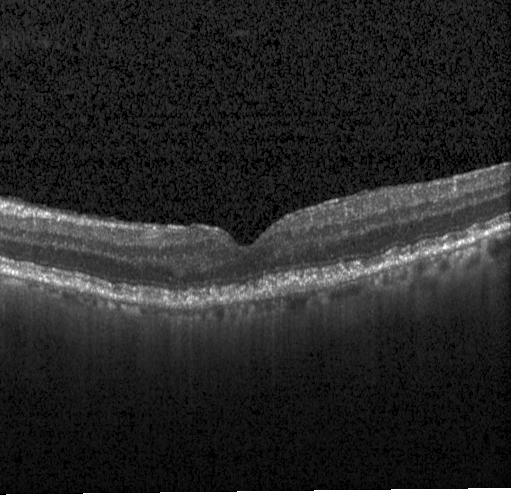
Centered on the fovea; optical coherence tomography scan; instrument: Heidelberg Spectralis — Dx: sub-RPE drusenoid deposits.